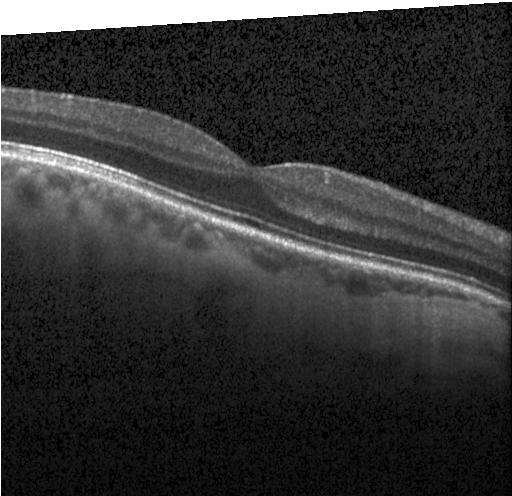

Retinal OCT cross-section — Neither CNV, DME, nor drusen.